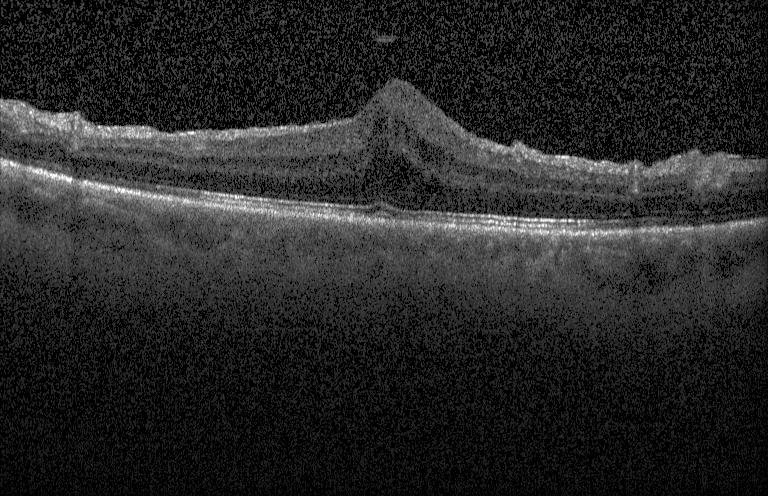

OCT line scan · spectral-domain optical coherence tomography · Heidelberg Spectralis OCT system
Impression: DME.